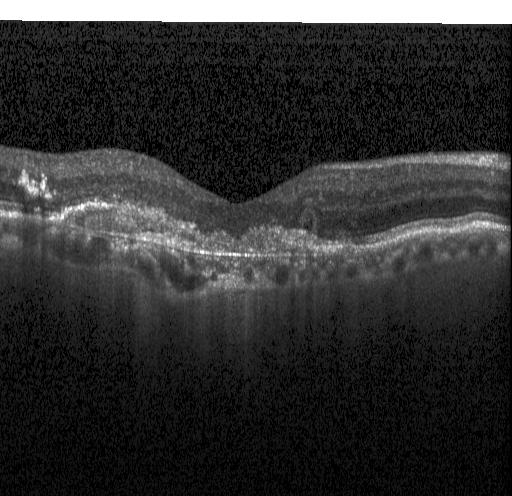 Finding: CNV.